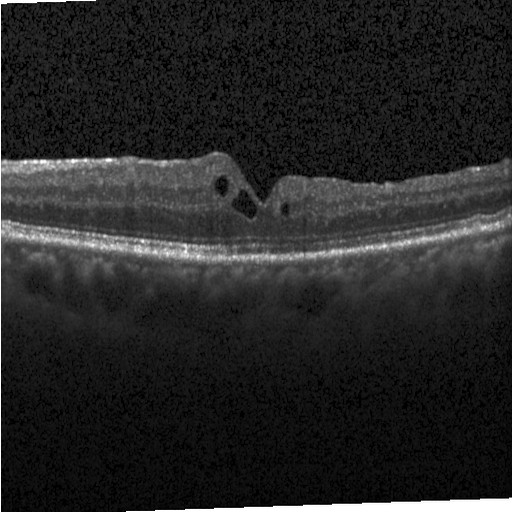 Dx: diabetic macular edema.